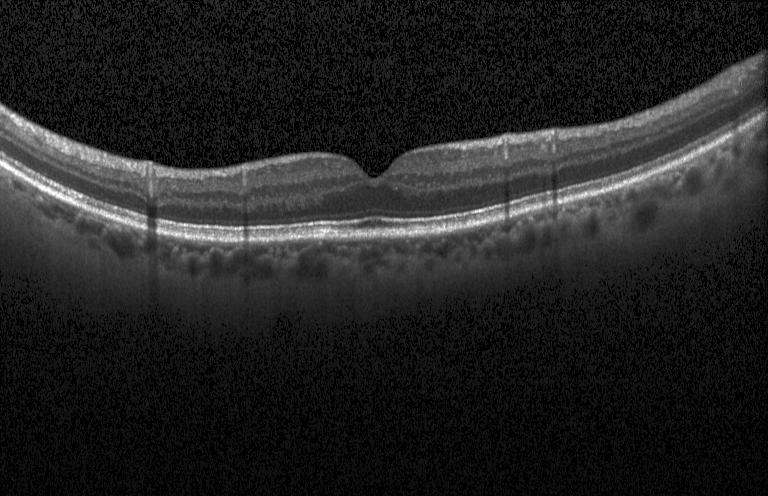
Diagnosis: no CNV, no DME, and no drusen.